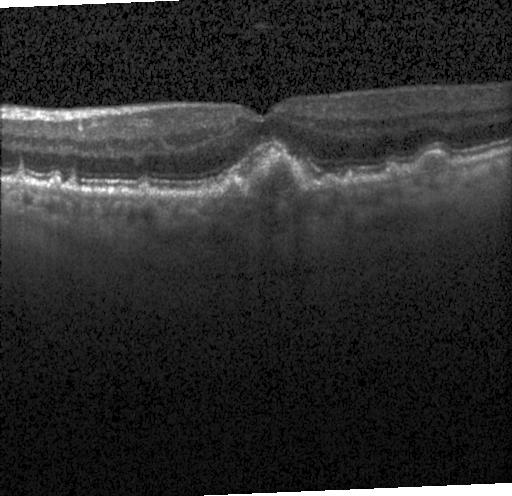
Spectral-domain OCT. OCT B-scan — A choroidal neovascular membrane.